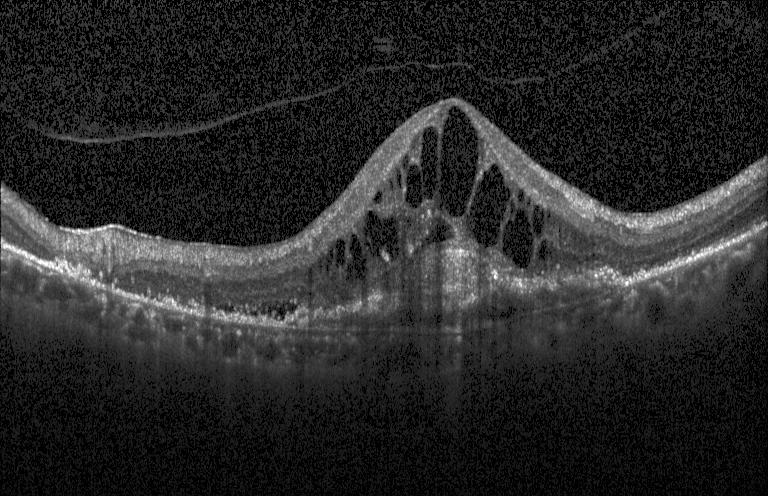

OCT line scan · centered on the fovea · spectral-domain OCT. Dx: CNV.